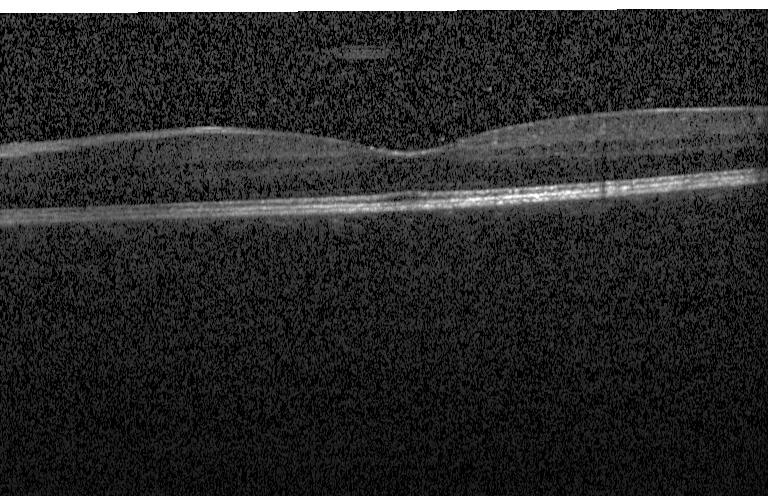

Retinal OCT B-scan, instrument: Heidelberg Spectralis, centered on the fovea — Impression: neither choroidal neovascularization, diabetic macular edema, nor drusen.